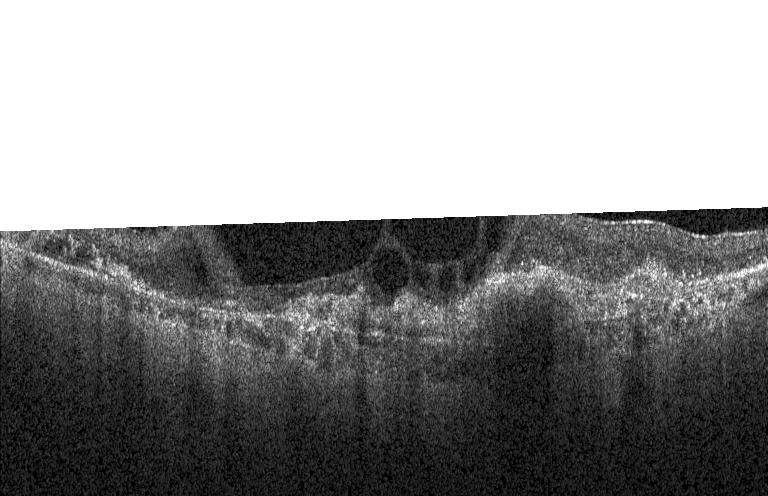 OCT B-scan — Finding: a choroidal neovascular membrane.